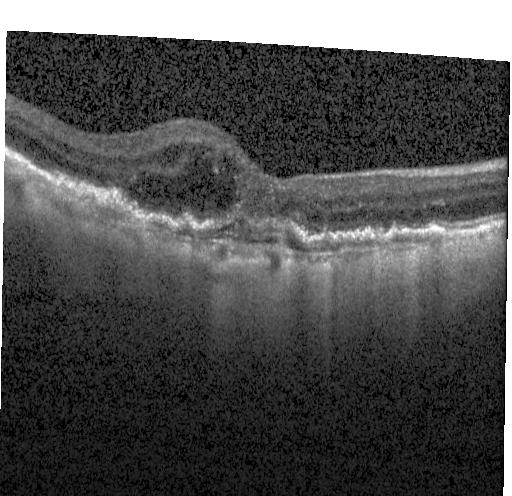
Optical coherence tomography B-scan; fovea-centered; Heidelberg Spectralis OCT system. Finding: a choroidal neovascular membrane.